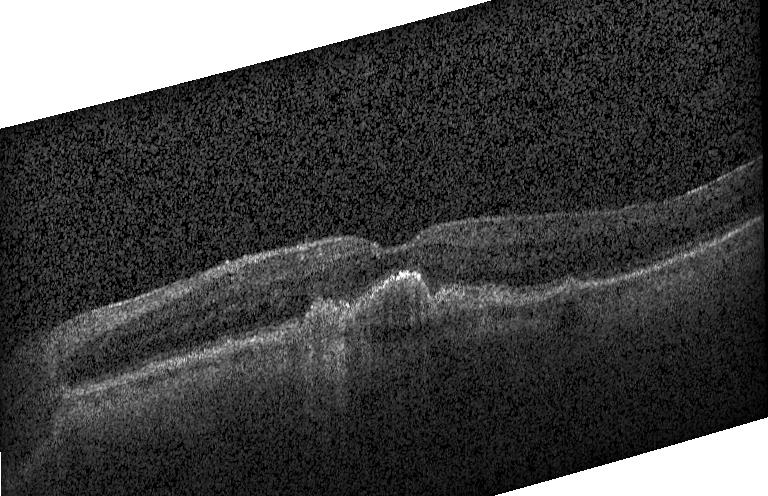

Instrument: Heidelberg Spectralis · retinal OCT B-scan. Choroidal neovascularization.